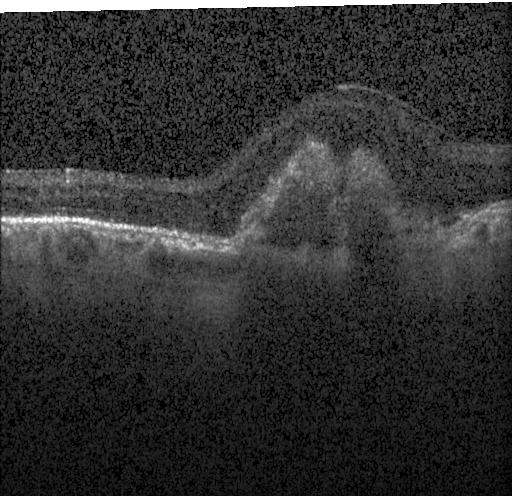

Fovea-centered. OCT line scan. Heidelberg Spectralis. The scan shows a choroidal neovascular membrane.